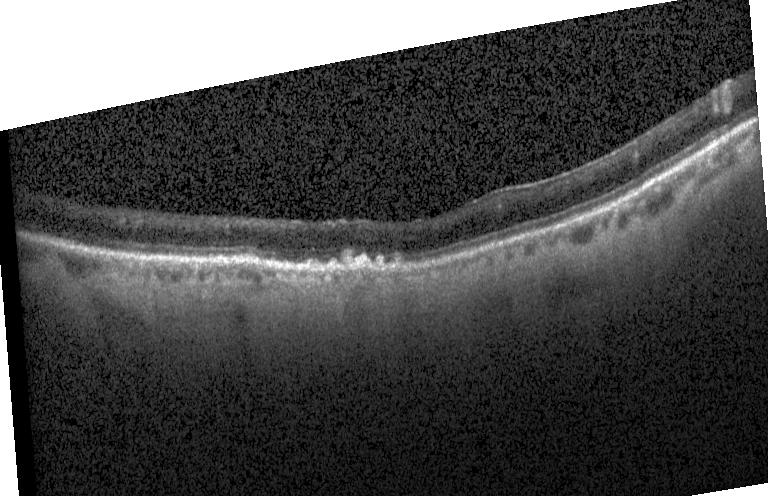
Retinal OCT cross-section; macular scan; spectral-domain optical coherence tomography; instrument: Heidelberg Spectralis.
Diagnosis: sub-RPE drusenoid deposits.